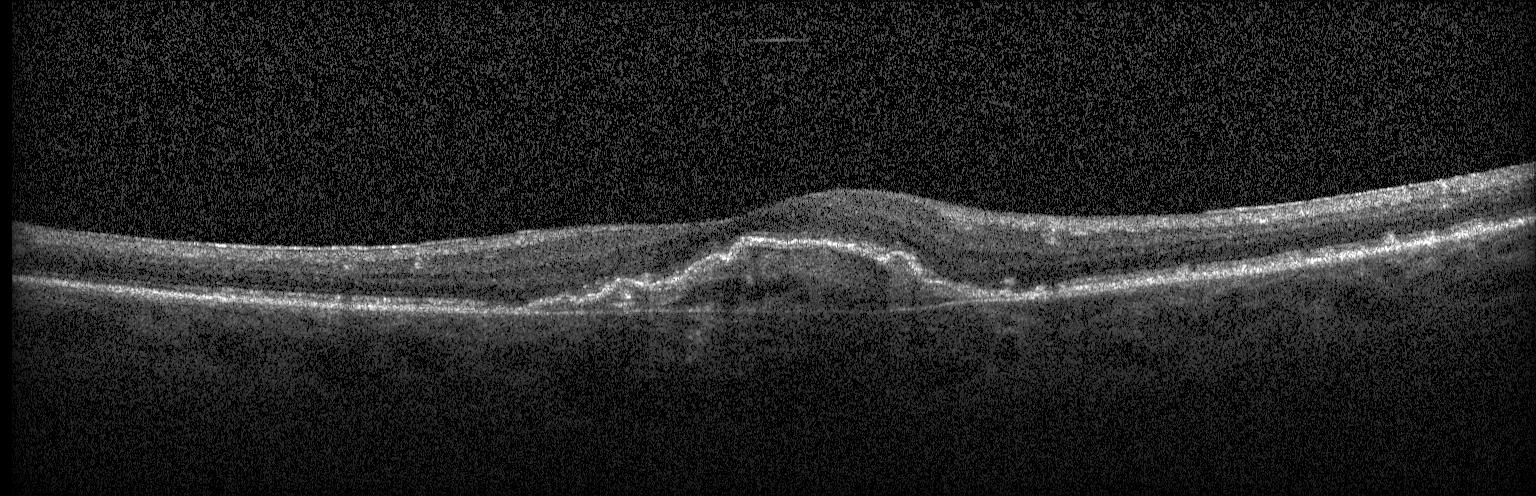

Impression: a choroidal neovascular membrane.